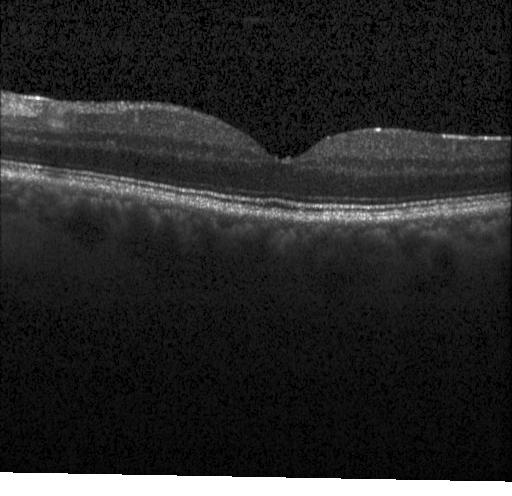 Diagnosis: no choroidal neovascularization, no diabetic macular edema, and no drusen.